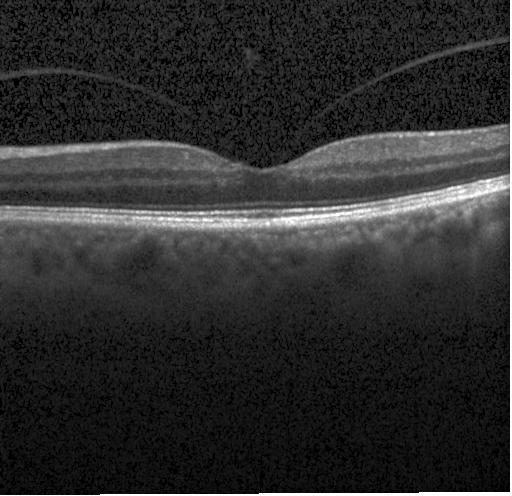
Macular OCT: no evidence of CNV, DME, or drusen.